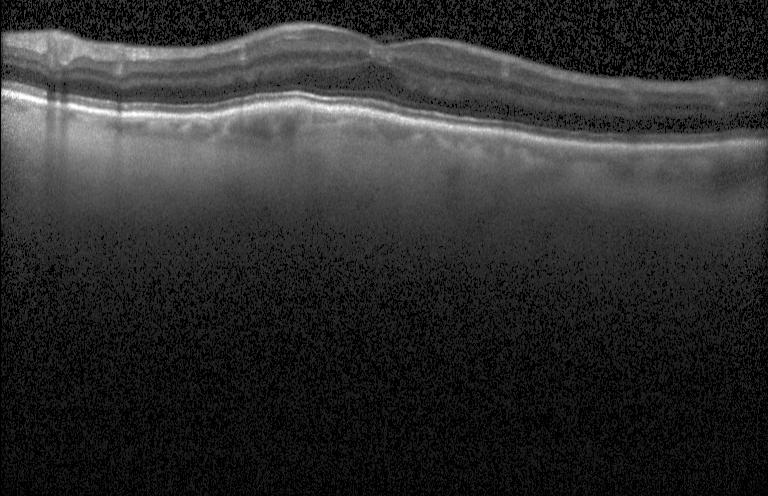
Finding: neither choroidal neovascularization, diabetic macular edema, nor drusen.